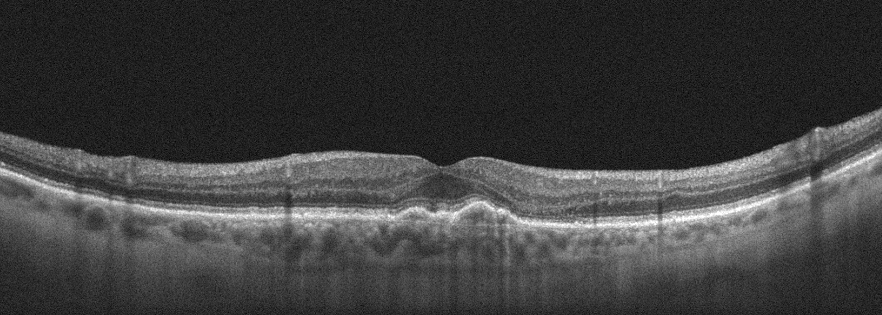

Finding: AMD.